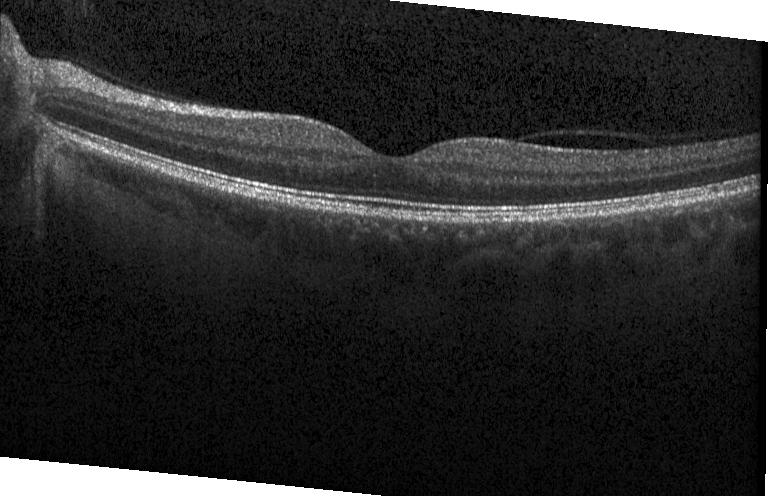 Macular OCT demonstrating no choroidal neovascularization, diabetic macular edema, or drusen.